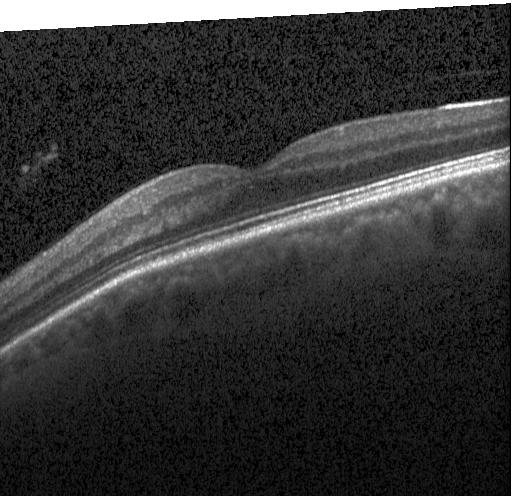 This B-scan demonstrates no choroidal neovascularization, diabetic macular edema, or drusen.